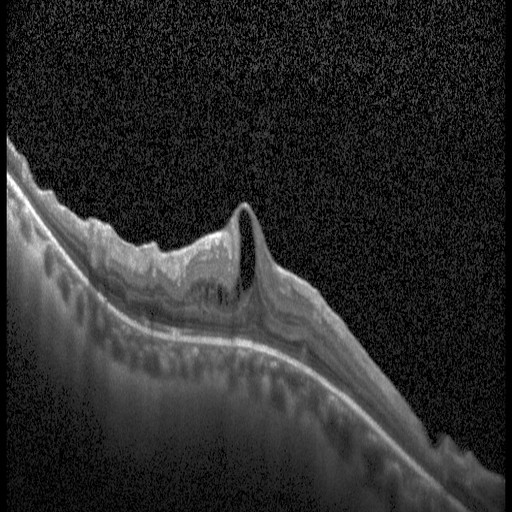
OCT B-scan, spectral-domain OCT, centered on the fovea
Dx: diabetic macular edema (DME).